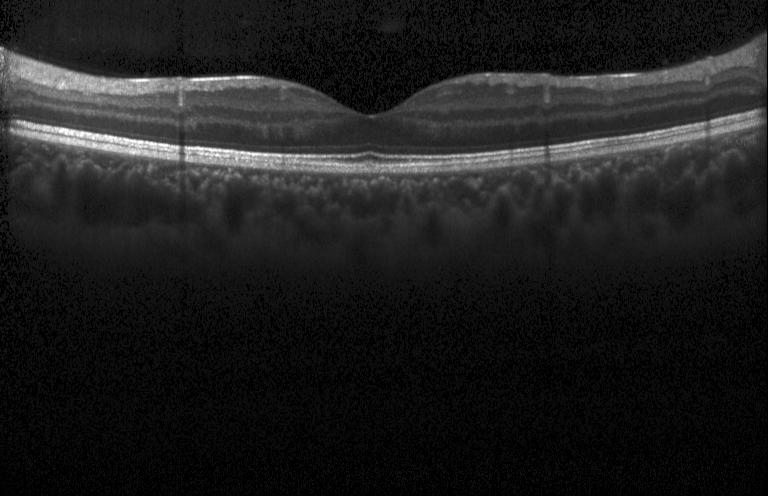

Through the macula, optical coherence tomography B-scan, Heidelberg Spectralis OCT system, spectral-domain optical coherence tomography — Diagnosis: neither choroidal neovascularization, diabetic macular edema, nor drusen.